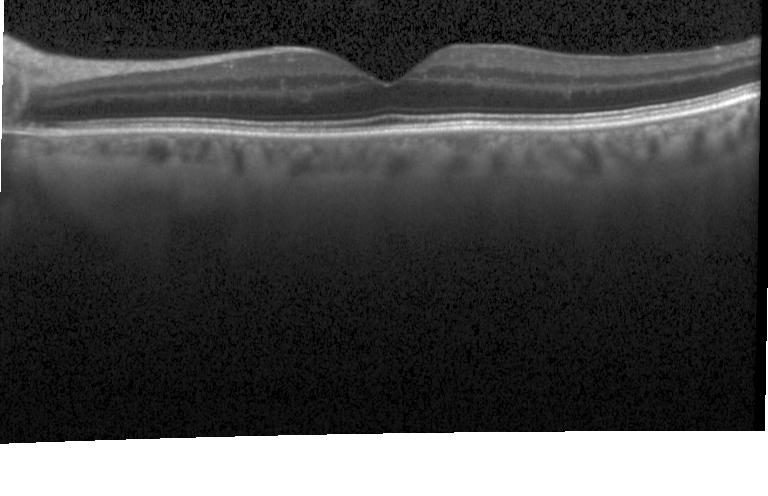 OCT B-scan
Finding: neither choroidal neovascularization, diabetic macular edema, nor drusen.